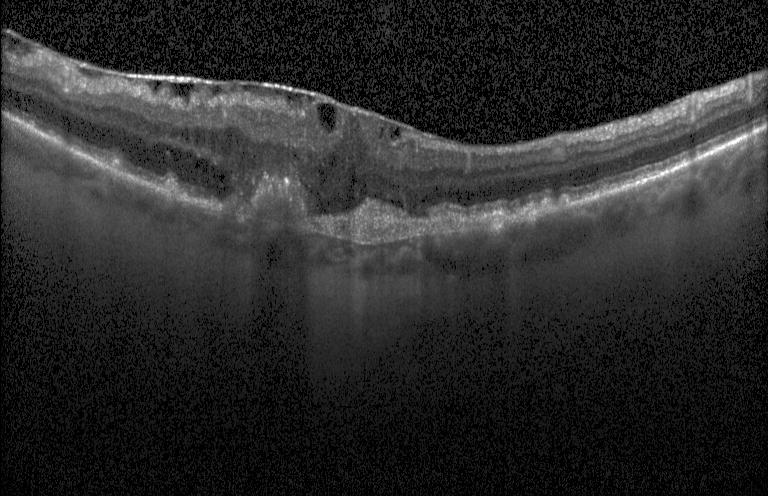
Macular OCT demonstrating a choroidal neovascular membrane.